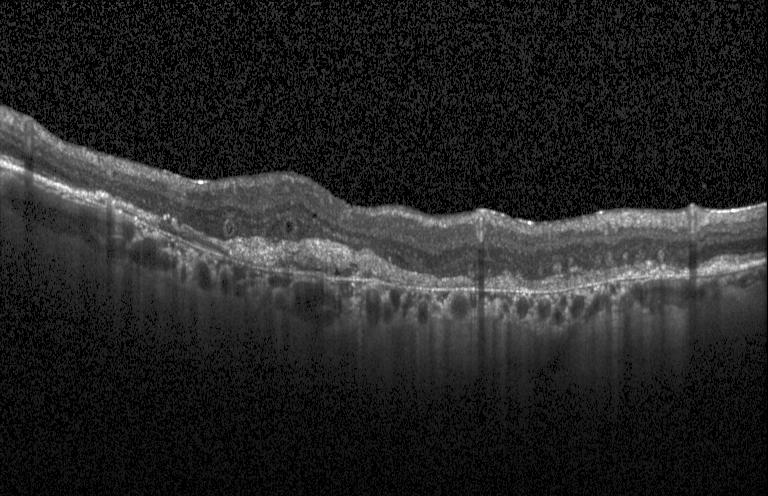
Assessment: a choroidal neovascular membrane.